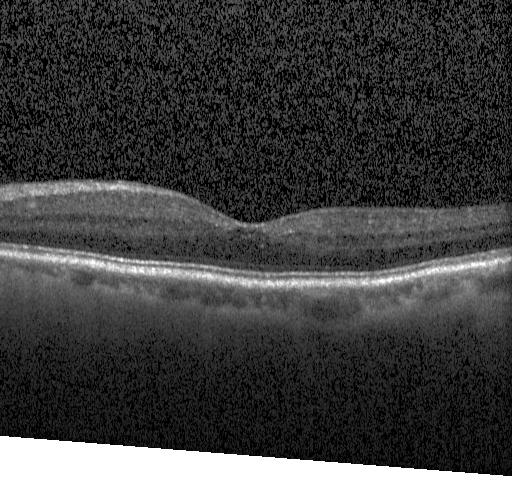
Finding: no evidence of choroidal neovascularization, diabetic macular edema, or drusen.